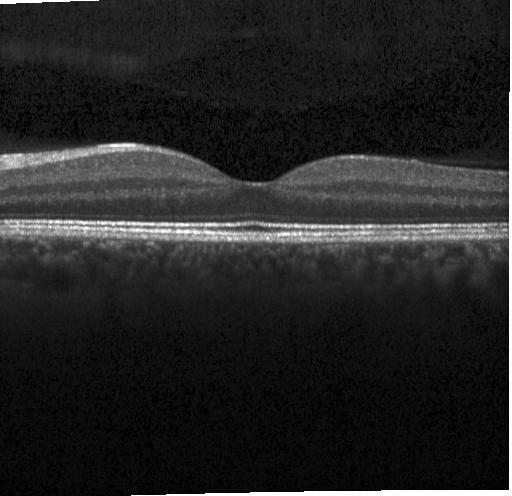 OCT line scan. Macular scan. Instrument: Heidelberg Spectralis — Finding: no choroidal neovascularization, diabetic macular edema, or drusen.